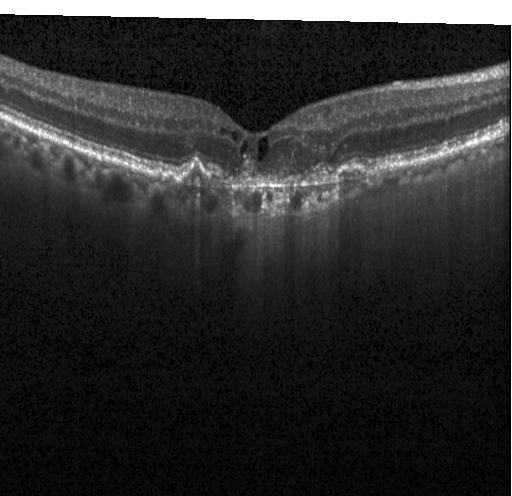
Macular scan · spectral-domain optical coherence tomography · instrument: Heidelberg Spectralis · retinal OCT B-scan.
Impression: choroidal neovascularization.